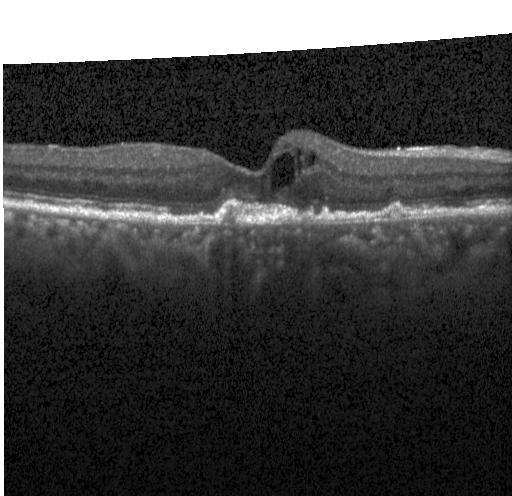 Spectral-domain OCT B-scan: choroidal neovascularization.